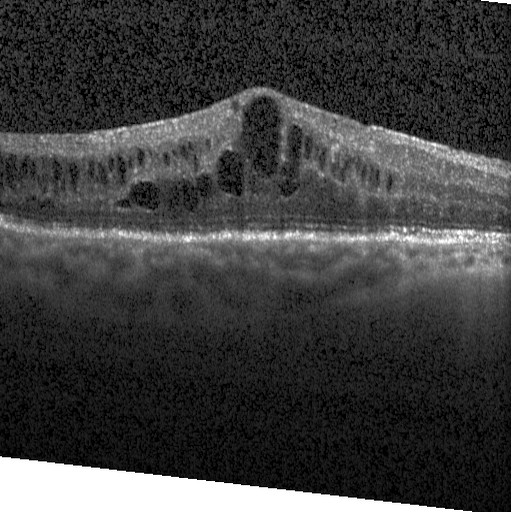
SD-OCT, centered on the fovea, Heidelberg Spectralis, OCT B-scan
Assessment: diabetic macular edema (DME).